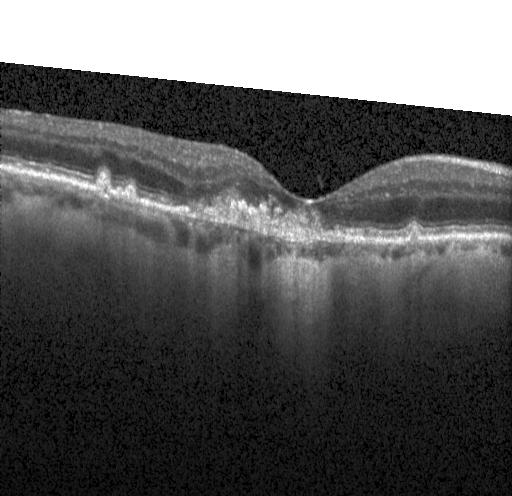
Dx: choroidal neovascularization.